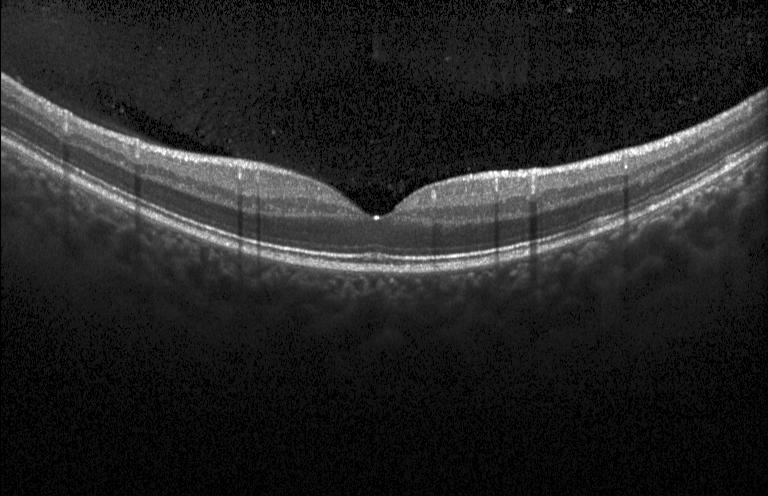

Finding: no CNV, DME, or drusen.